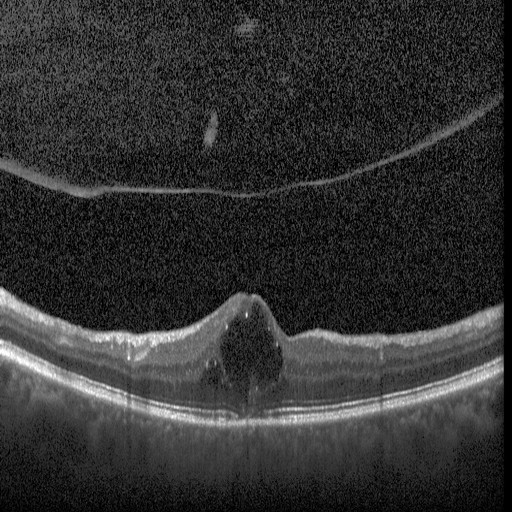
OCT B-scan · acquired on a Heidelberg Spectralis.
Assessment: diabetic macular edema.